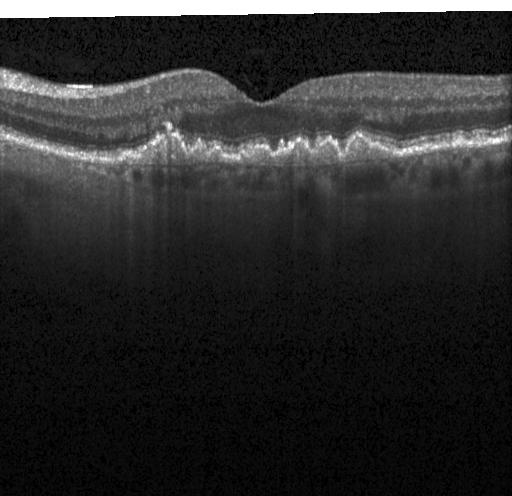 Horizontal scan through the fovea; OCT B-scan; acquired on a Heidelberg Spectralis.
OCT finding: multiple drusen.